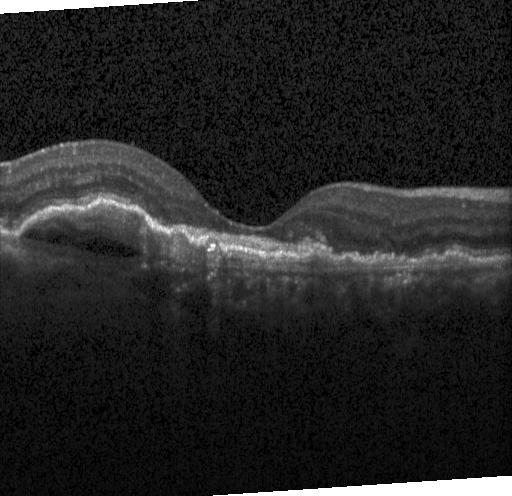 Heidelberg Spectralis. Optical coherence tomography B-scan. SD-OCT. Fovea-centered.
Diagnosis: a choroidal neovascular membrane.